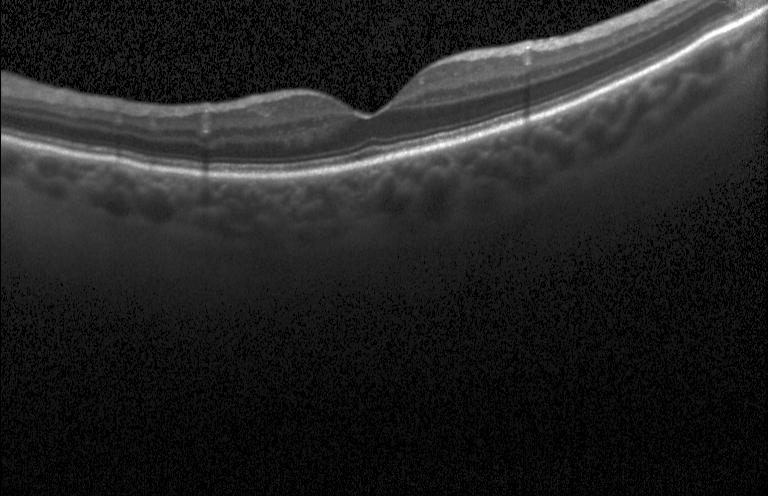
Optical coherence tomography scan
OCT finding: neither choroidal neovascularization, diabetic macular edema, nor drusen.